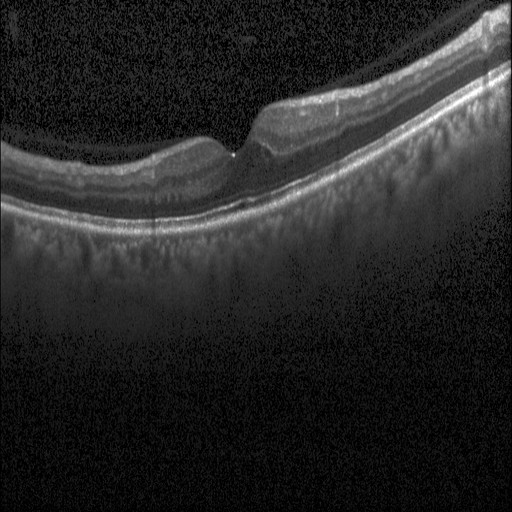 Spectral-domain optical coherence tomography · optical coherence tomography scan
Diabetic macular edema.